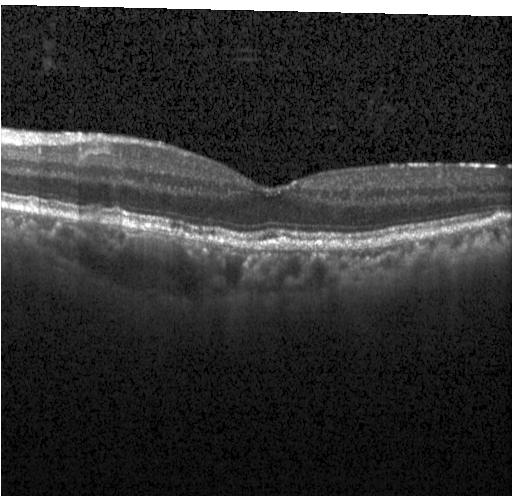
Finding: drusen.